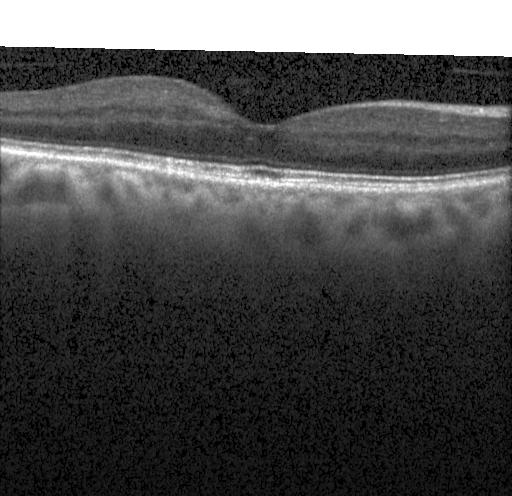

Spectral-domain optical coherence tomography. Optical coherence tomography scan. Heidelberg Spectralis OCT system.
Assessment: neither choroidal neovascularization, diabetic macular edema, nor drusen.